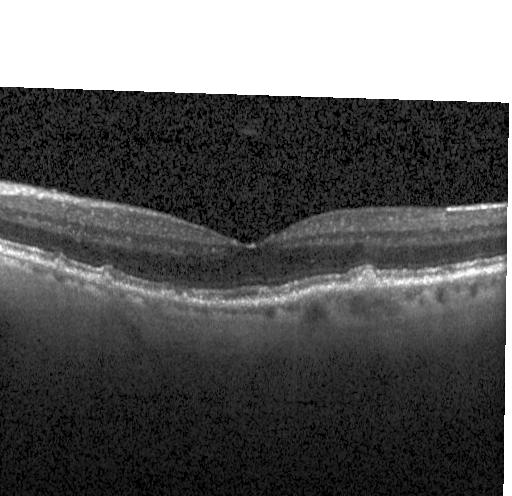 OCT B-scan. Finding: drusen.